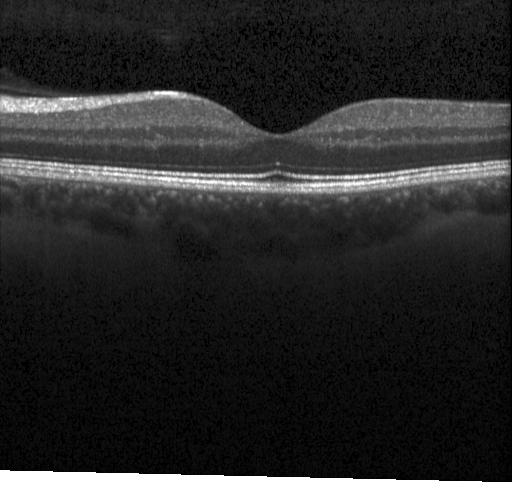 Retinal OCT cross-section showing no CNV, no DME, and no drusen.